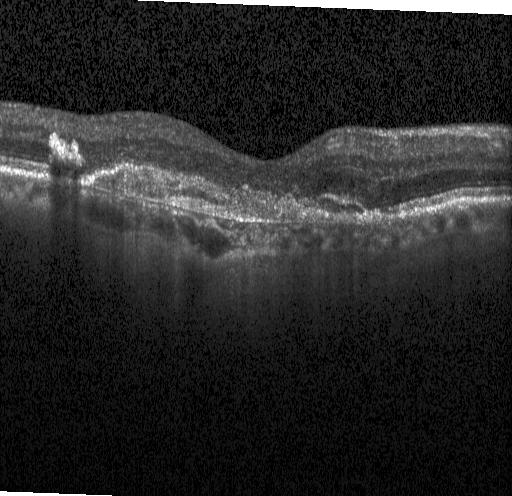

Spectral-domain optical coherence tomography, optical coherence tomography B-scan
Impression: a choroidal neovascular membrane.